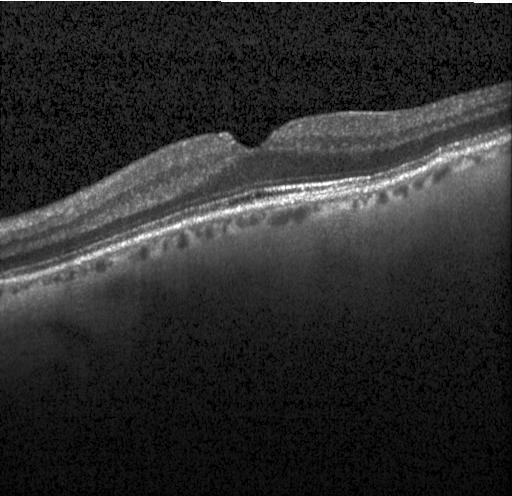 OCT B-scan showing no CNV, DME, or drusen.